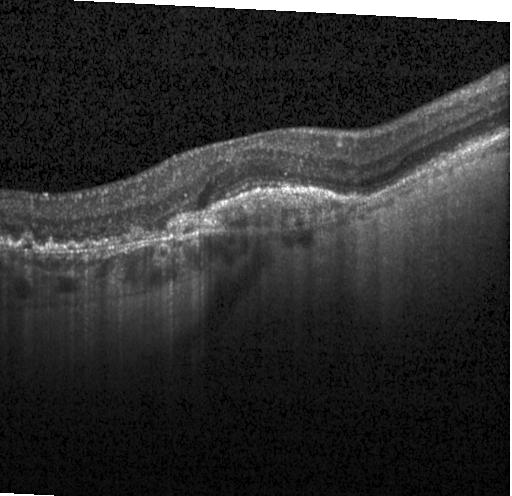 This B-scan demonstrates a choroidal neovascular membrane.